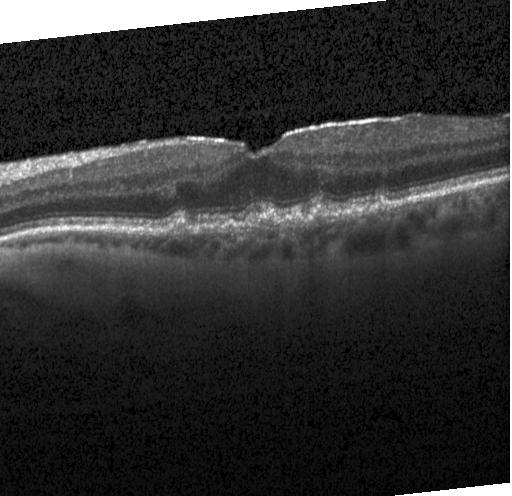
Optical coherence tomography scan. Heidelberg Spectralis OCT system. Spectral-domain optical coherence tomography. Through the macula — This B-scan demonstrates drusen.